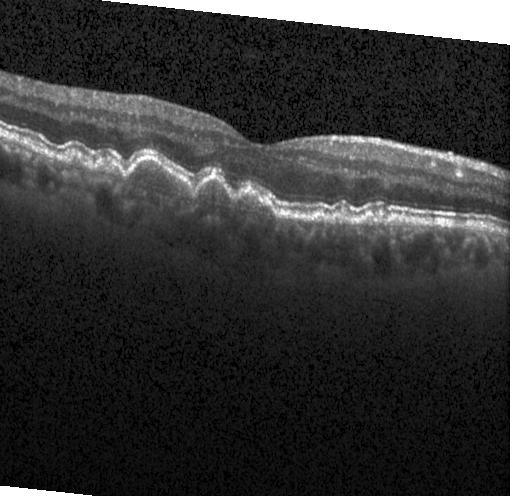
Acquired on a Heidelberg Spectralis · optical coherence tomography B-scan — Diagnosis: sub-RPE drusenoid deposits.